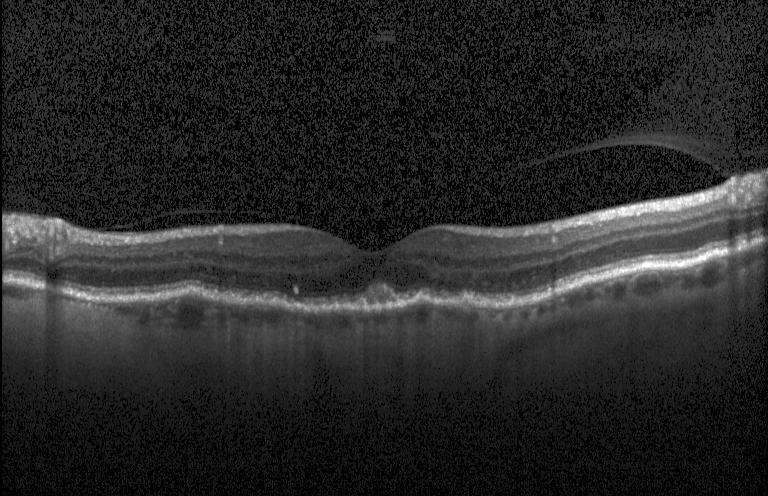 Macular OCT: drusen.